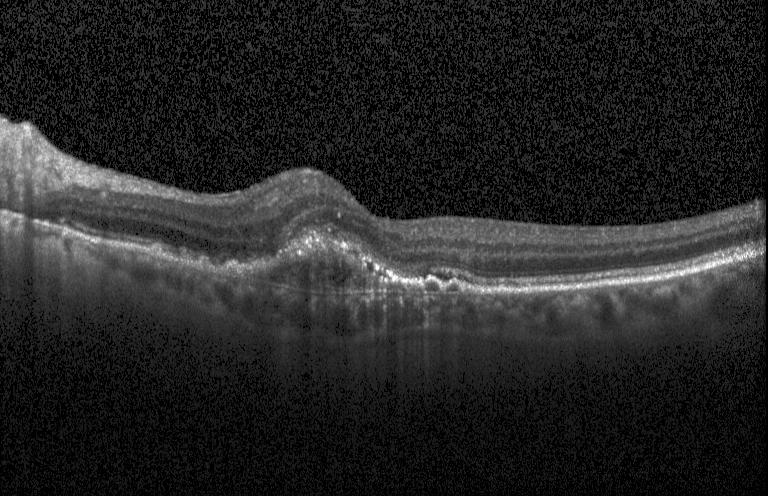
Optical coherence tomography scan
Diagnosis: a choroidal neovascular membrane.